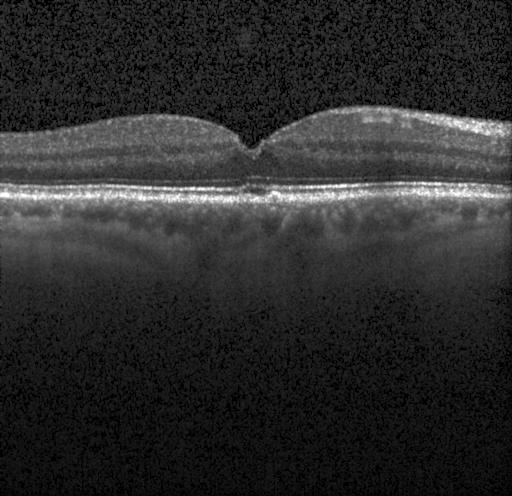
Dx: sub-RPE drusenoid deposits.